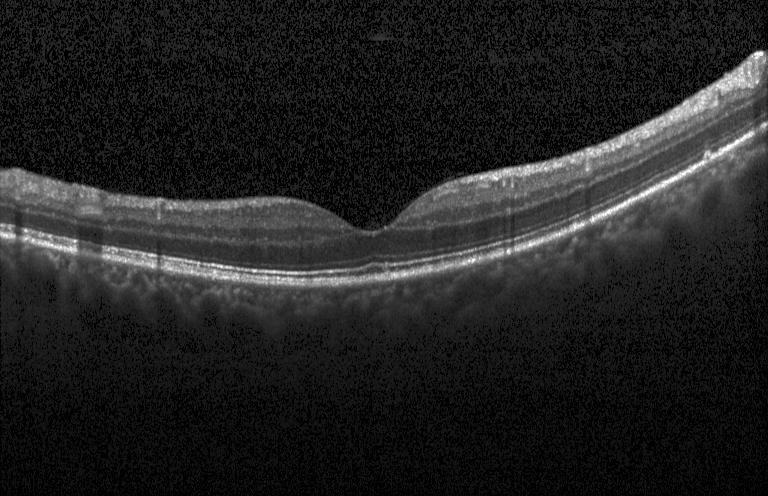 Instrument: Heidelberg Spectralis. Fovea-centered. SD-OCT. Retinal OCT cross-section.
Impression: no evidence of CNV, DME, or drusen.